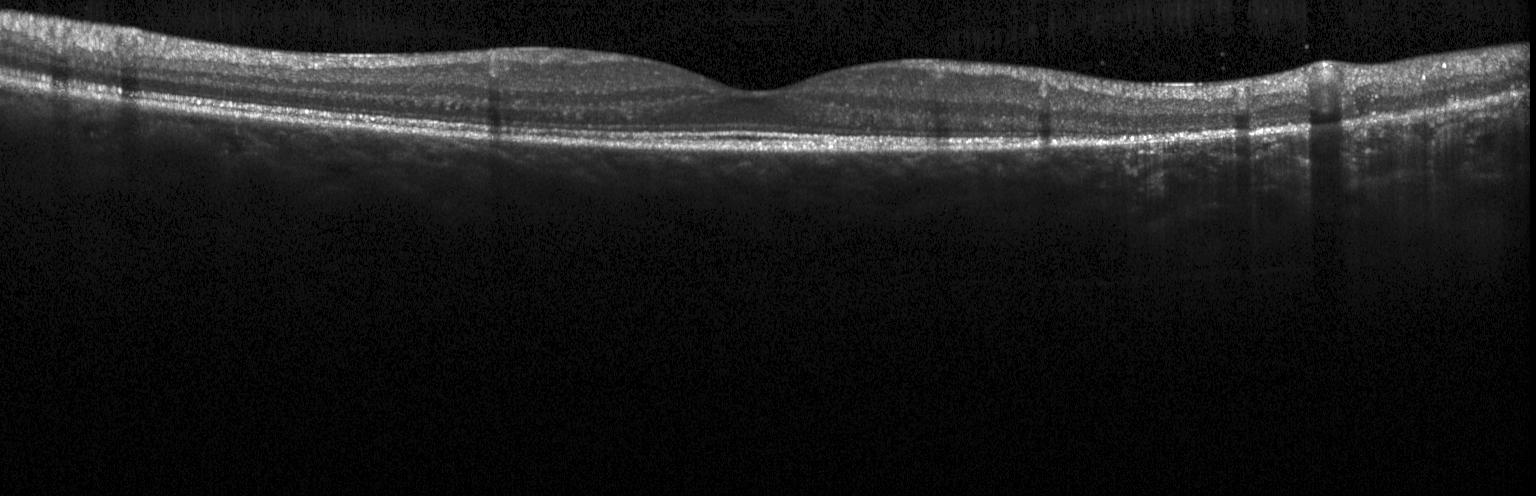

SD-OCT. Retinal OCT cross-section. Impression: no evidence of choroidal neovascularization, diabetic macular edema, or drusen.